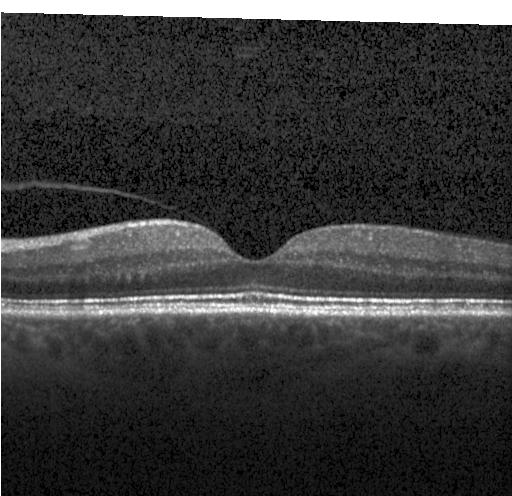 OCT line scan.
No choroidal neovascularization, no diabetic macular edema, and no drusen.